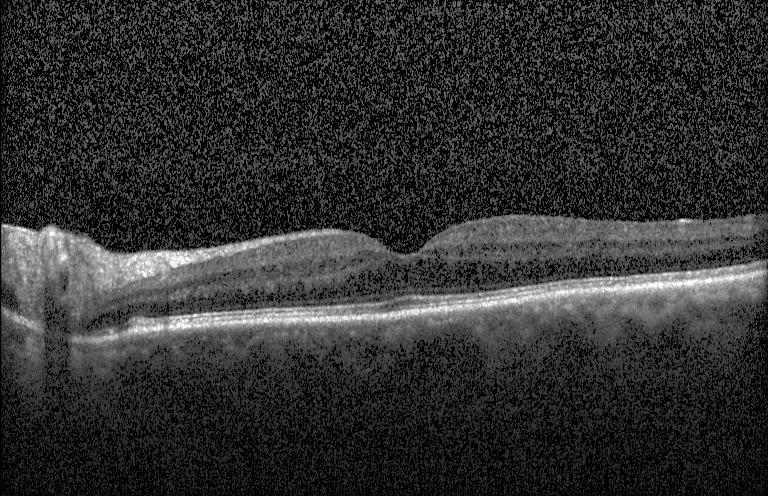
Through the macula, retinal OCT cross-section, Heidelberg Spectralis, spectral-domain optical coherence tomography
Impression: no evidence of CNV, DME, or drusen.